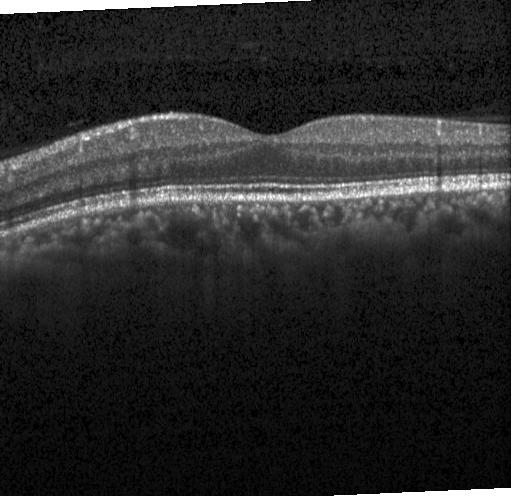
Dx: no evidence of choroidal neovascularization, diabetic macular edema, or drusen.